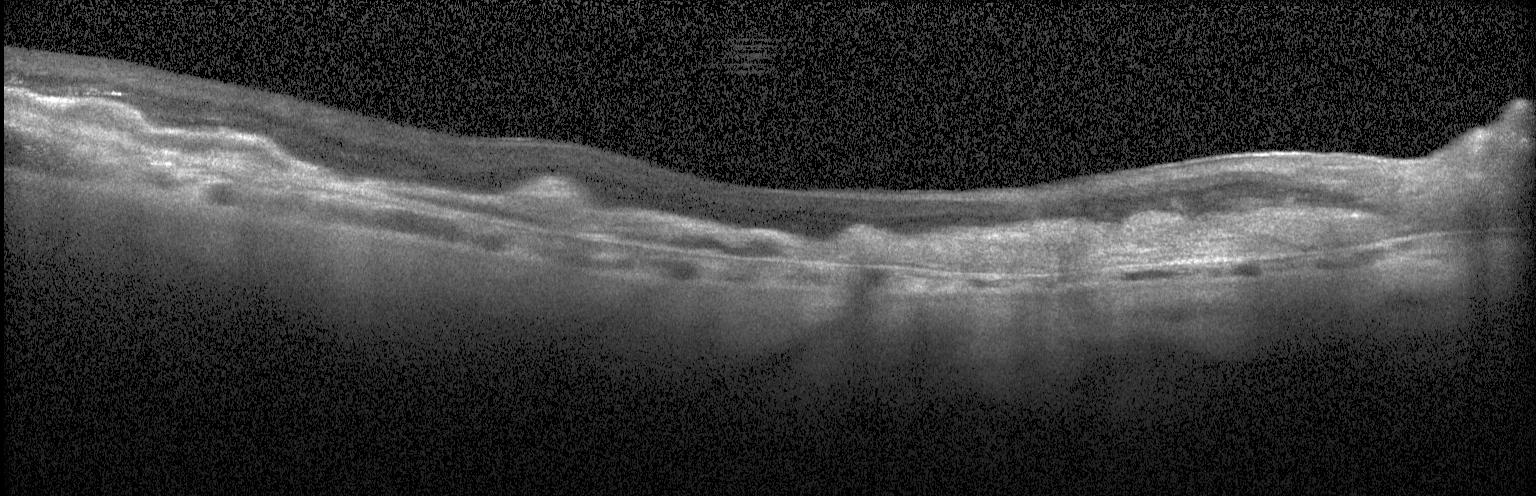

Spectral-domain OCT, optical coherence tomography B-scan
Dx: choroidal neovascularization.